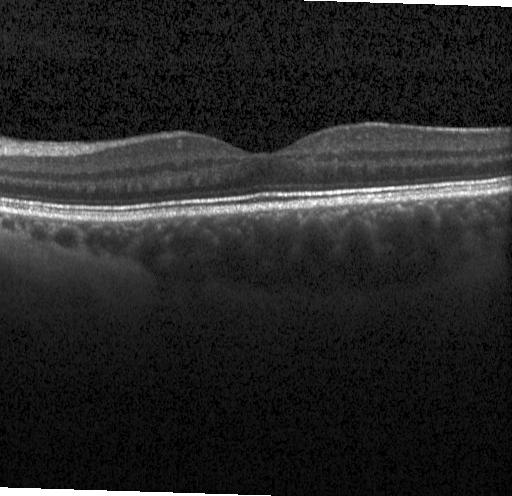

Optical coherence tomography scan. Dx: neither choroidal neovascularization, diabetic macular edema, nor drusen.